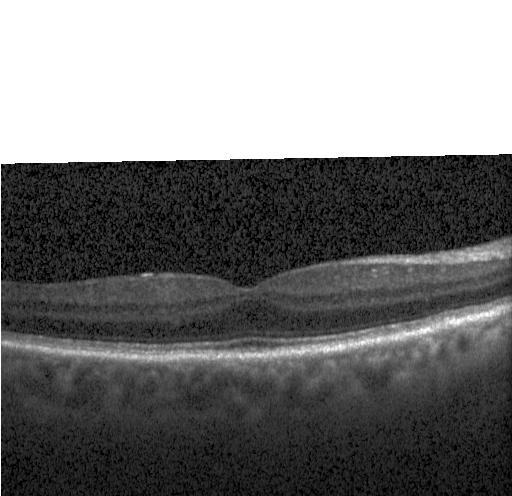

Acquired on a Heidelberg Spectralis, retinal OCT cross-section, fovea-centered.
Dx: no evidence of CNV, DME, or drusen.